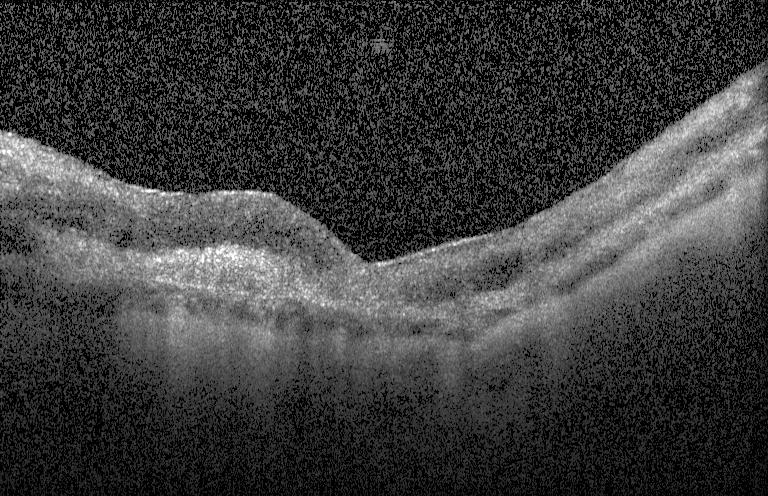
OCT B-scan. Spectral-domain OCT. Heidelberg Spectralis
Impression: choroidal neovascularization.